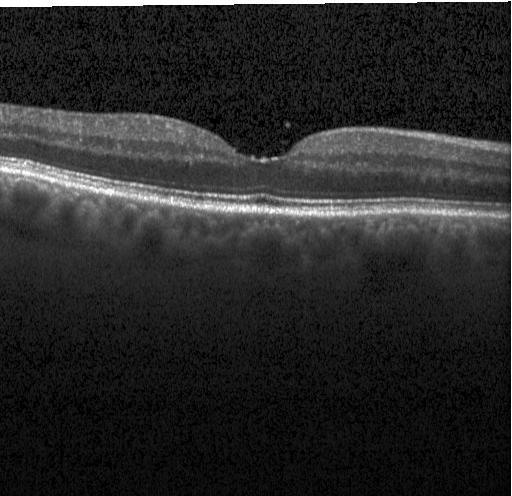
Retinal OCT cross-section showing no choroidal neovascularization, diabetic macular edema, or drusen.